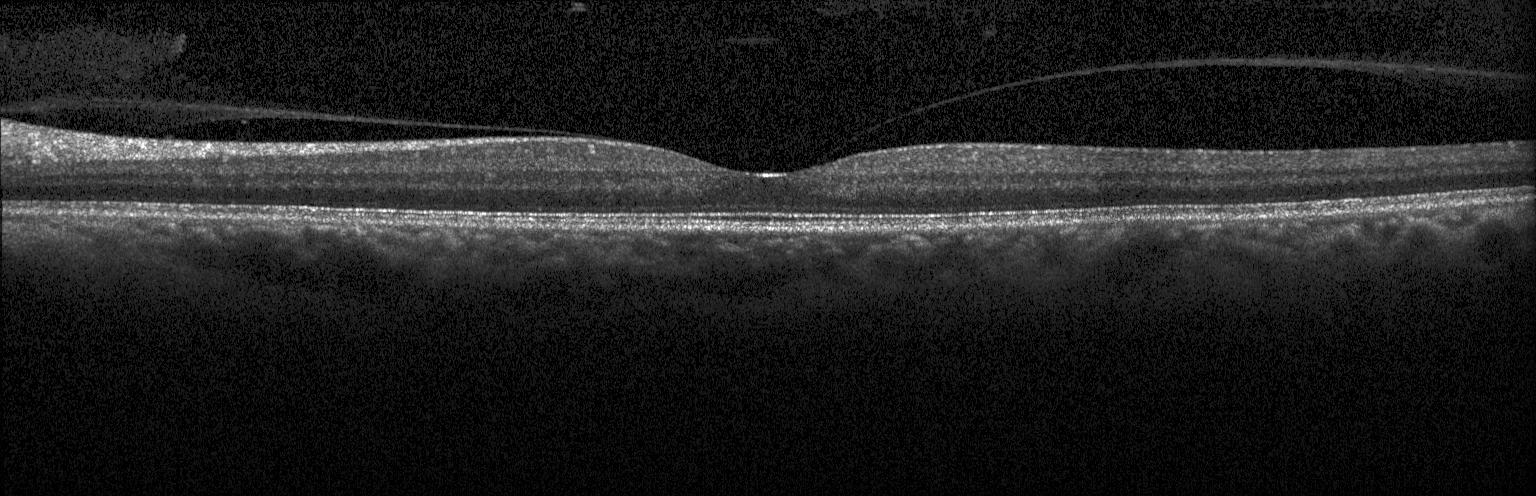

Retinal OCT B-scan, fovea-centered, spectral-domain OCT, Heidelberg Spectralis.
Dx: no evidence of CNV, DME, or drusen.